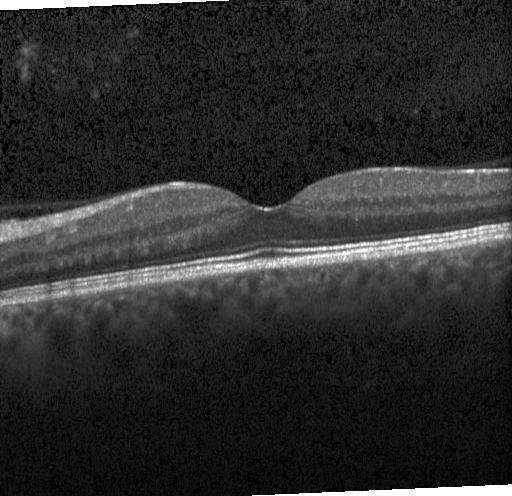 Heidelberg Spectralis OCT system, horizontal scan through the fovea, spectral-domain OCT, OCT B-scan. Dx: neither CNV, DME, nor drusen.